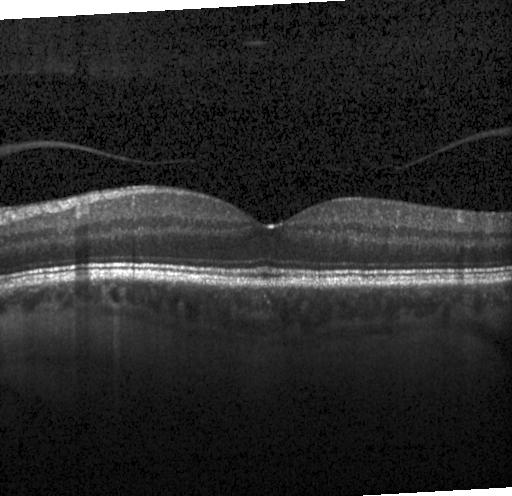 Retinal OCT cross-section; through the macula — Dx: no evidence of CNV, DME, or drusen.